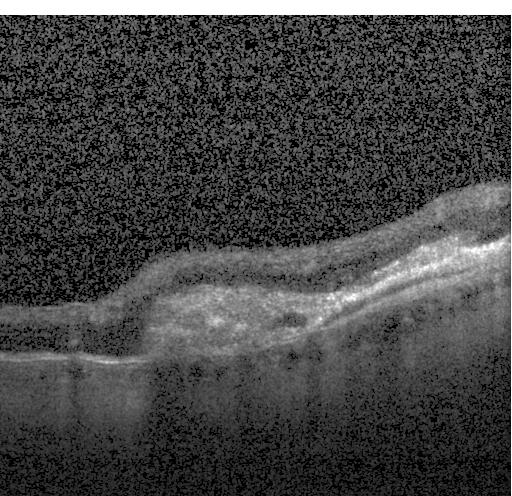 Instrument: Heidelberg Spectralis. SD-OCT. Retinal OCT cross-section. Horizontal scan through the fovea — Macular OCT: a choroidal neovascular membrane.